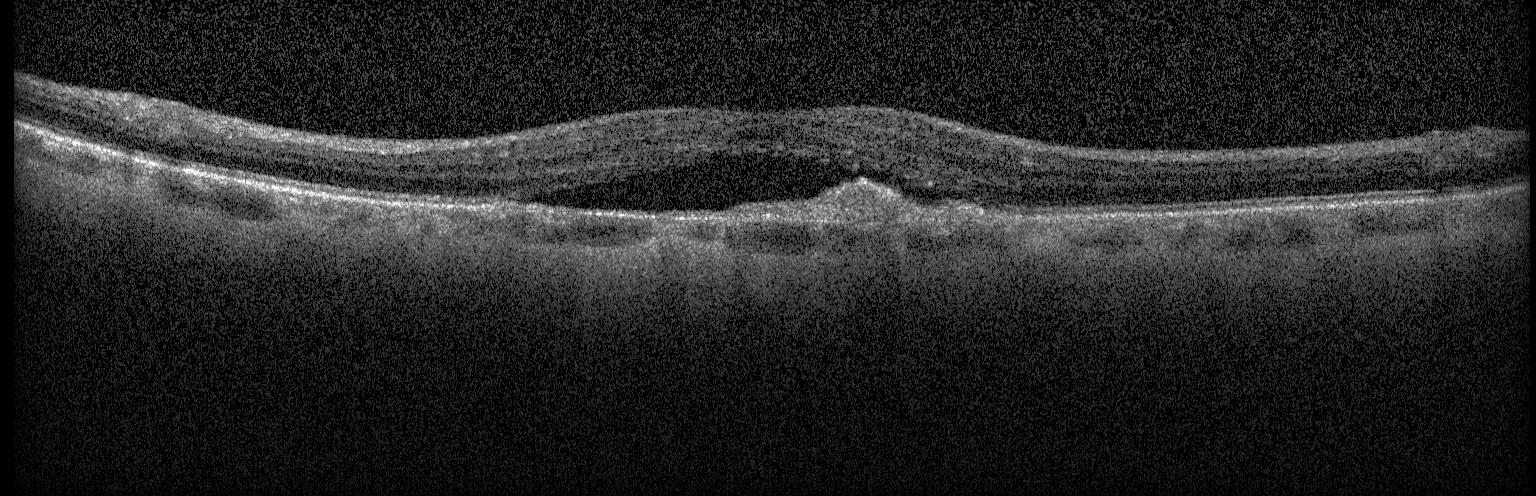
Retinal OCT cross-section showing choroidal neovascularization.